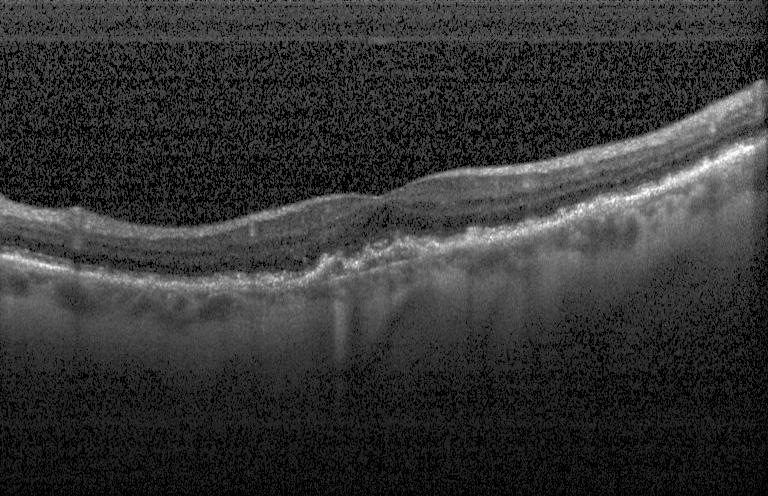
The scan shows a choroidal neovascular membrane.